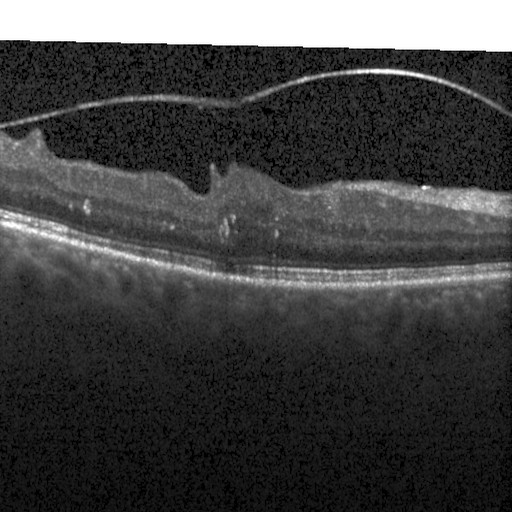 Spectral-domain optical coherence tomography; OCT B-scan
Macular OCT: diabetic macular edema (DME).